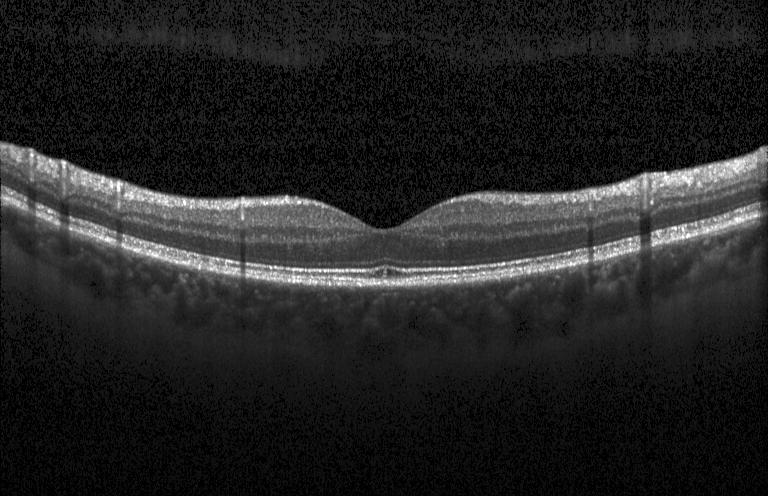

Impression: no CNV, no DME, and no drusen.